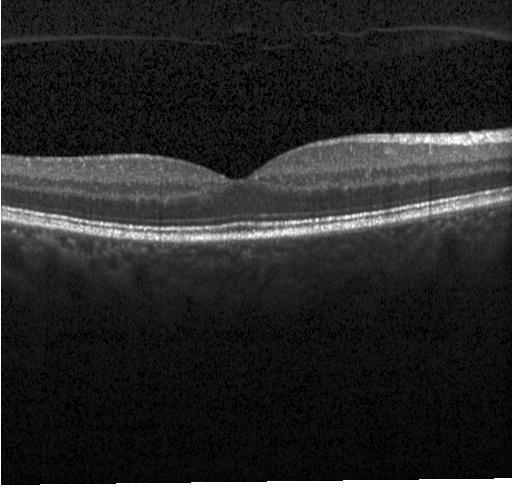 Optical coherence tomography B-scan · through the macula. OCT finding: no evidence of choroidal neovascularization, diabetic macular edema, or drusen.